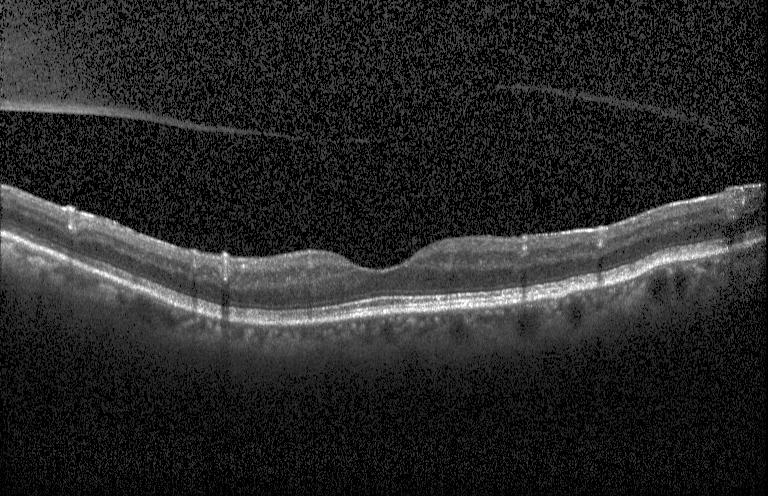

Assessment: no evidence of CNV, DME, or drusen.